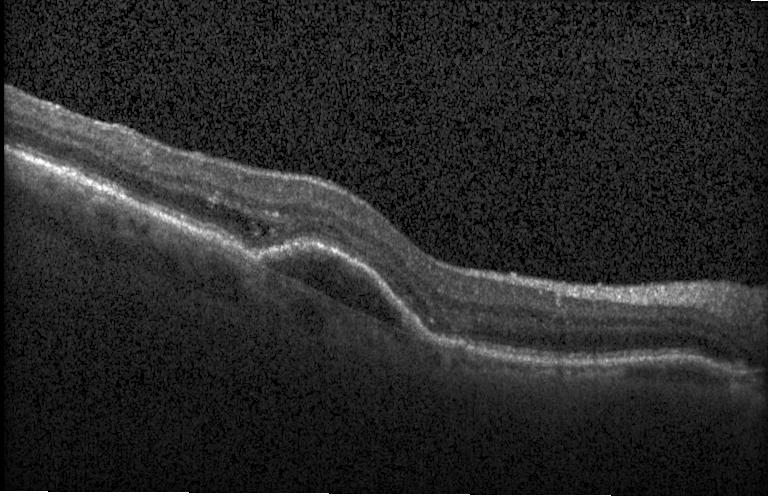
Macular OCT demonstrating CNV.